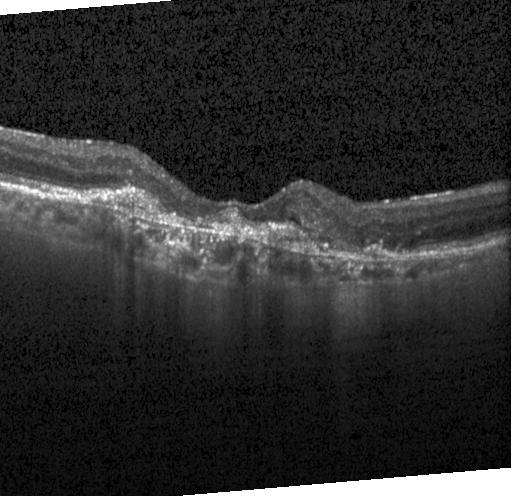

OCT line scan
This B-scan demonstrates a choroidal neovascular membrane.